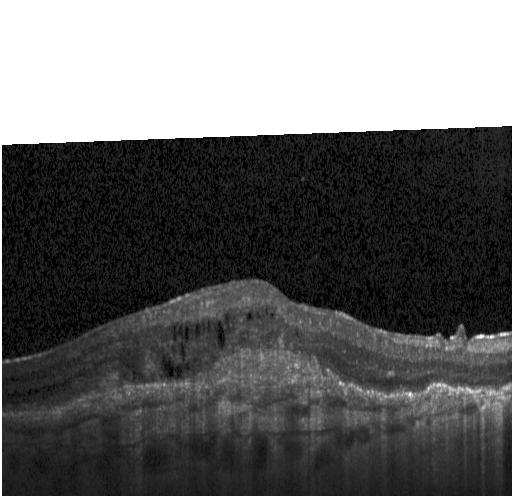 Macular scan; retinal OCT B-scan; Heidelberg Spectralis.
Diagnosis: a choroidal neovascular membrane.